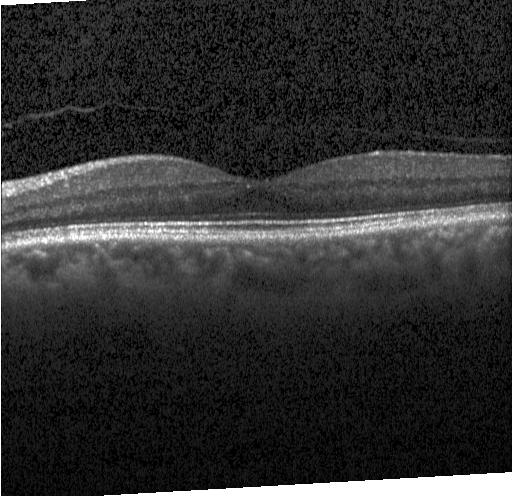

Diagnosis: no CNV, no DME, and no drusen.